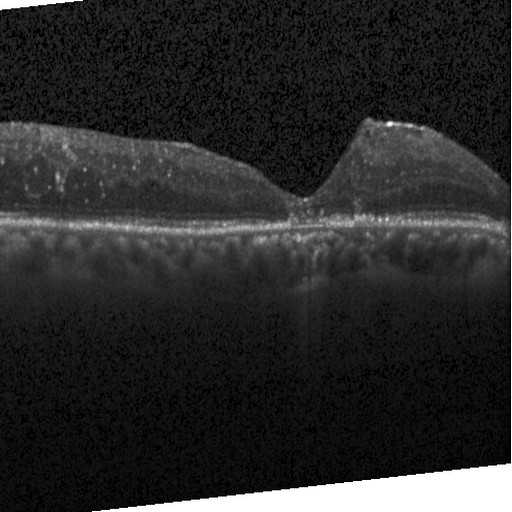
Dx: diabetic macular edema.